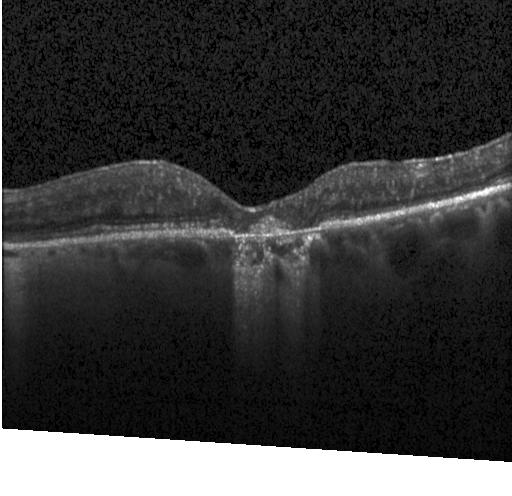

Retinal OCT B-scan. Horizontal scan through the fovea. Instrument: Heidelberg Spectralis
Assessment: CNV.